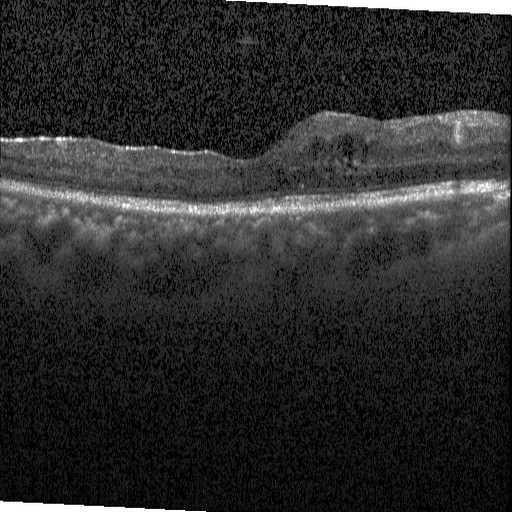

Finding: diabetic macular edema (DME).